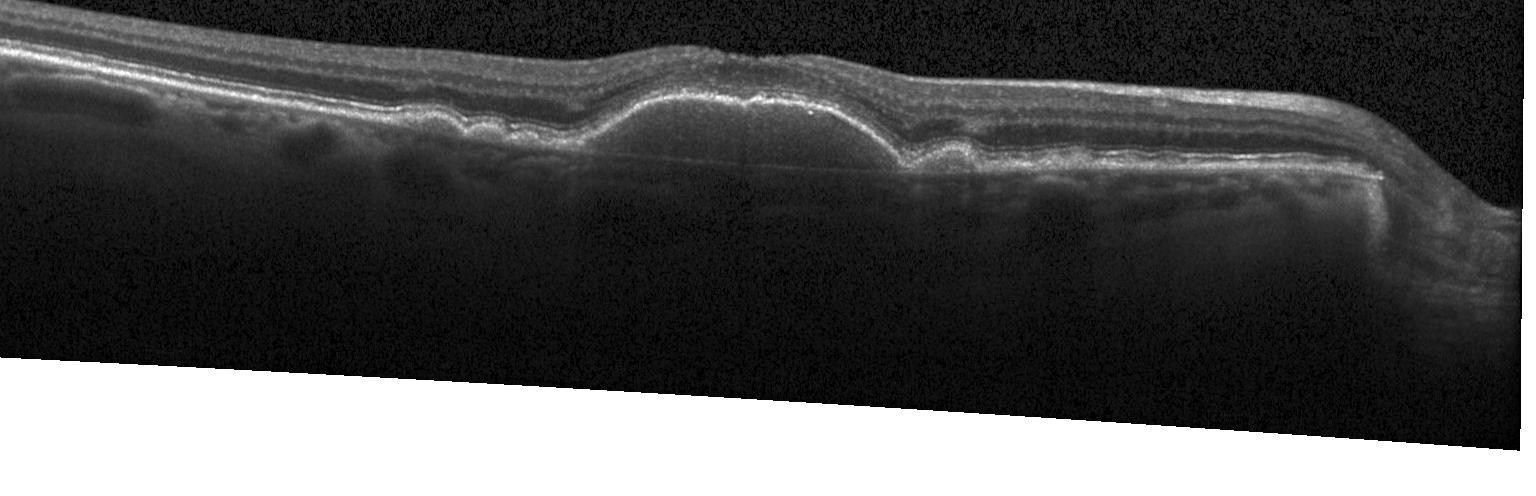

OCT B-scan. Horizontal scan through the fovea. Instrument: Heidelberg Spectralis. Spectral-domain optical coherence tomography. This B-scan demonstrates a choroidal neovascular membrane.